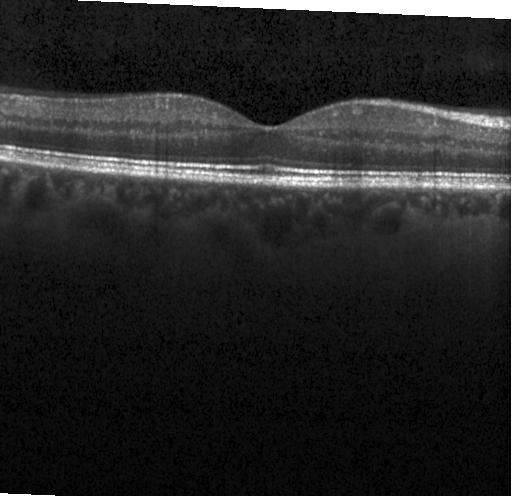
Macular OCT: no choroidal neovascularization, diabetic macular edema, or drusen.